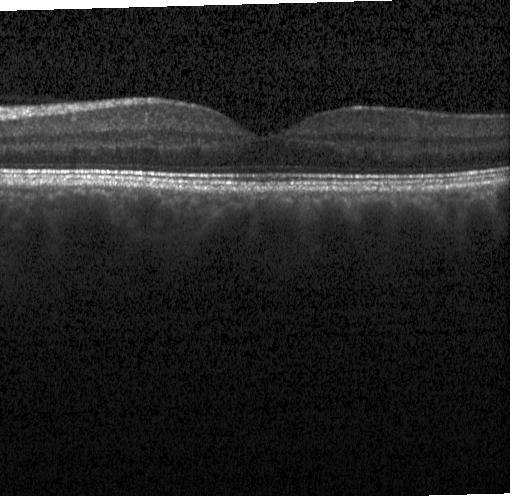

Heidelberg Spectralis; retinal OCT cross-section; fovea-centered.
Impression: no CNV, DME, or drusen.